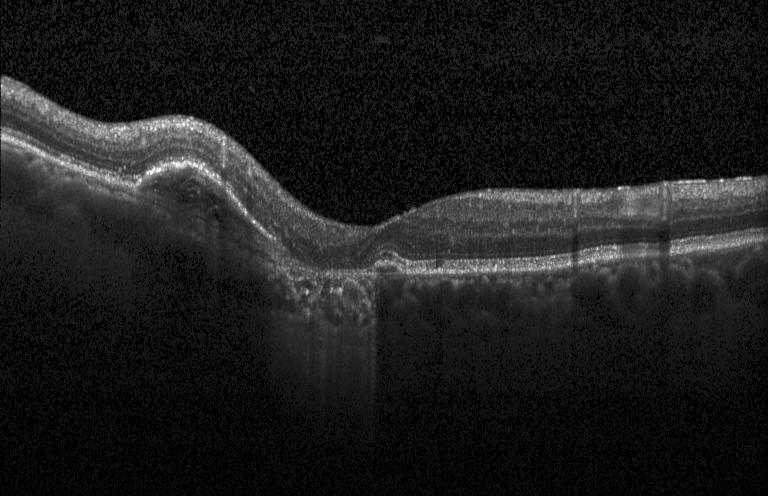 Centered on the fovea, OCT line scan.
Assessment: choroidal neovascularization.